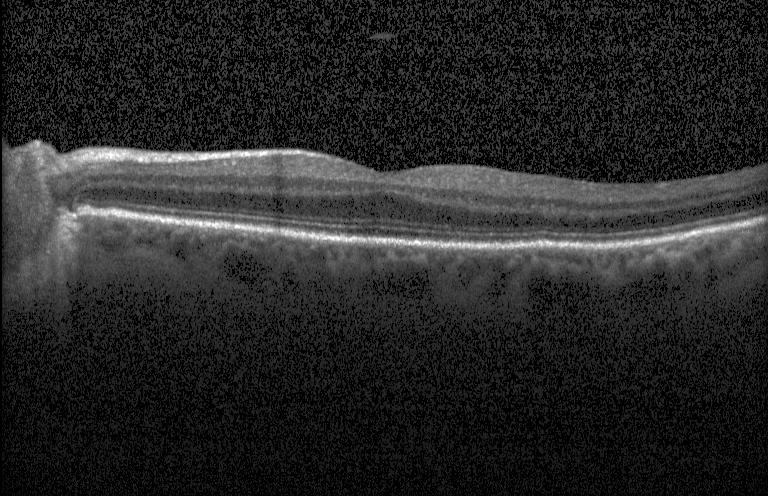 Retinal OCT cross-section; through the macula; spectral-domain optical coherence tomography; acquired on a Heidelberg Spectralis.
Finding: no CNV, no DME, and no drusen.